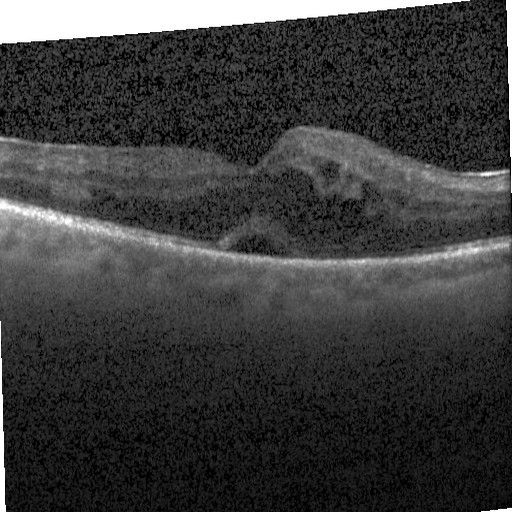

The scan shows diabetic macular edema.